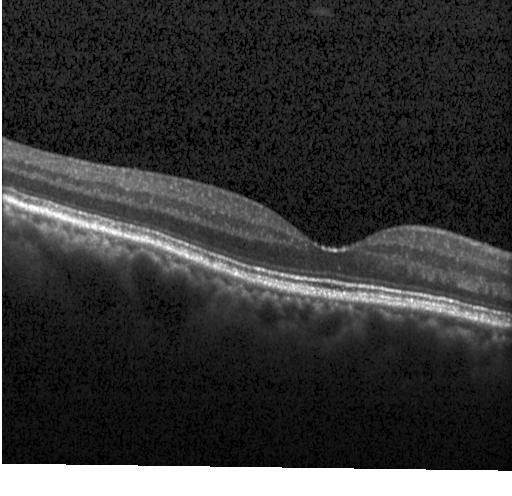 No choroidal neovascularization, diabetic macular edema, or drusen.